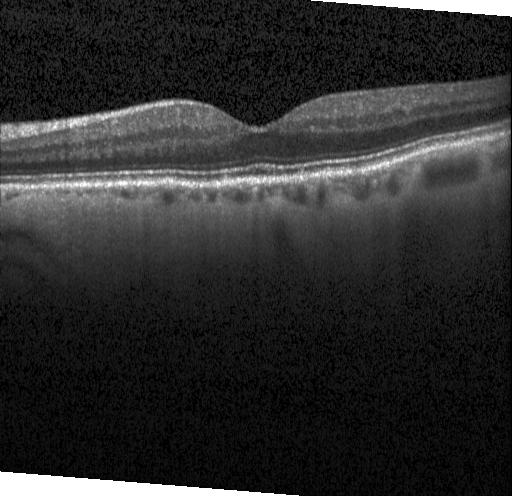 OCT line scan.
Impression: no CNV, DME, or drusen.